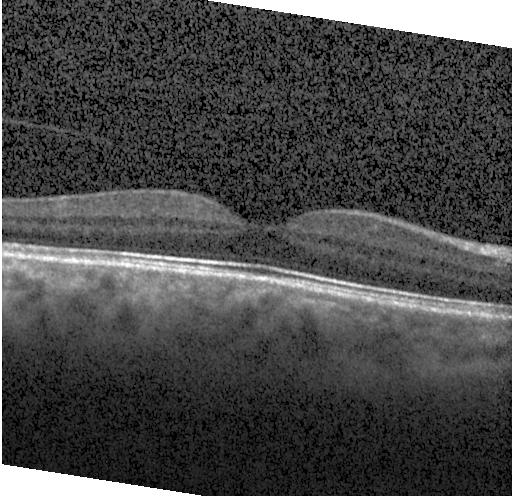
Optical coherence tomography B-scan · spectral-domain optical coherence tomography. Diagnosis: no evidence of choroidal neovascularization, diabetic macular edema, or drusen.